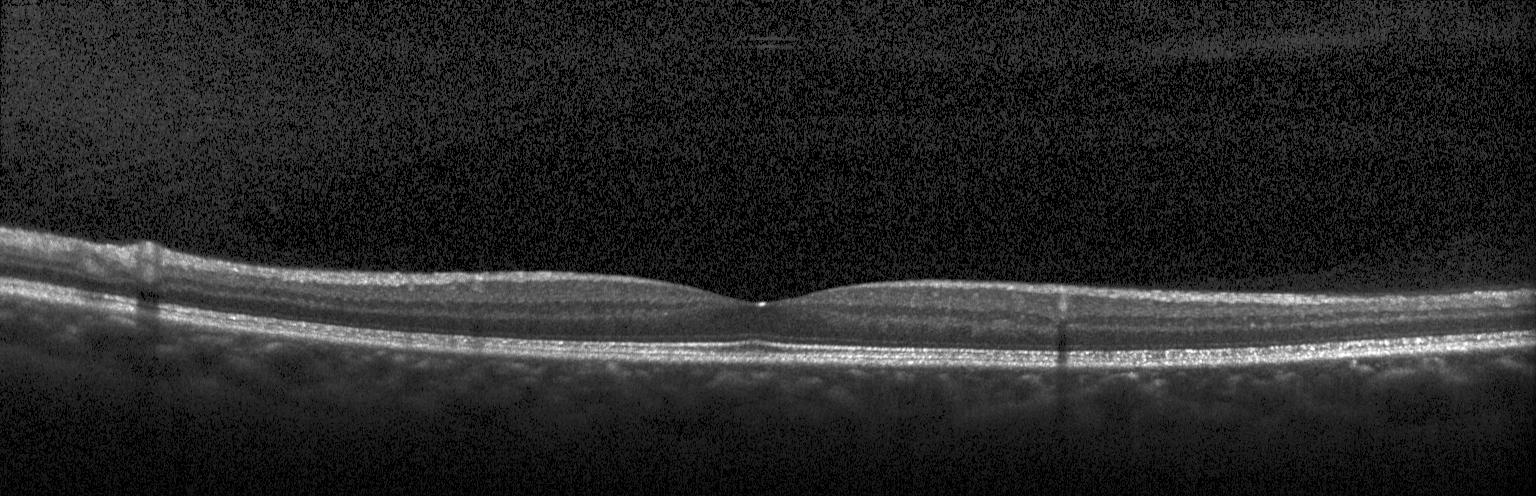

Horizontal scan through the fovea, OCT B-scan
Impression: neither CNV, DME, nor drusen.